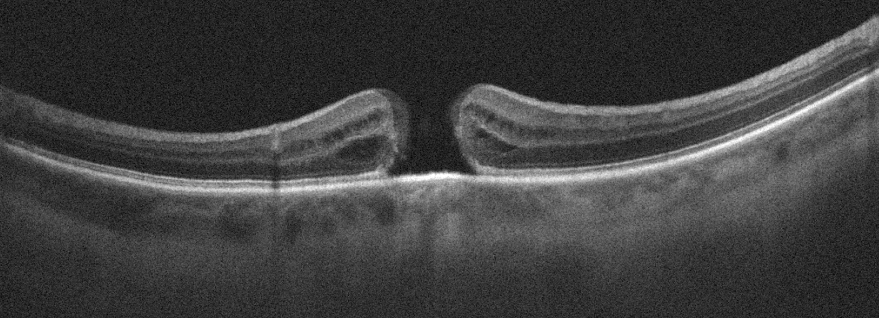
Retinal OCT cross-section.
Vitreomacular interface disease.